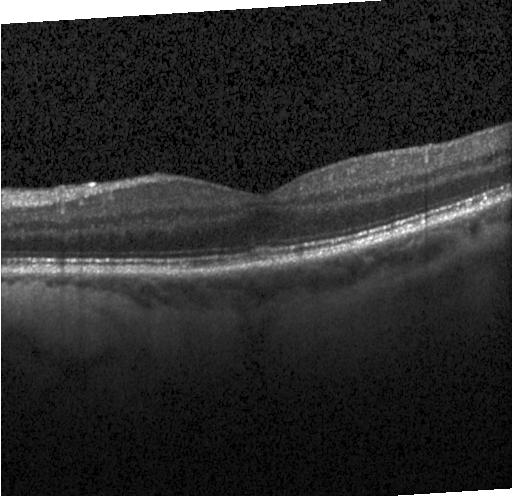
OCT line scan — No evidence of choroidal neovascularization, diabetic macular edema, or drusen.